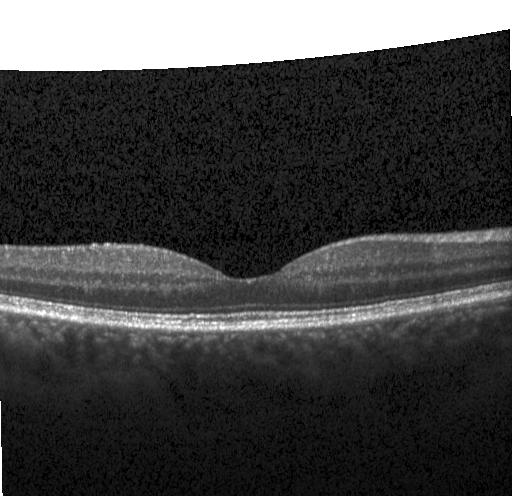
Instrument: Heidelberg Spectralis, retinal OCT cross-section, spectral-domain optical coherence tomography
Diagnosis: no CNV, no DME, and no drusen.